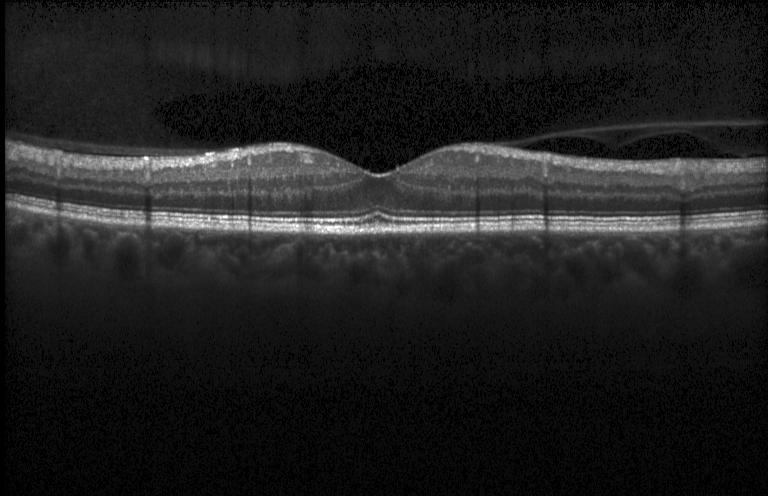

Assessment: no choroidal neovascularization, no diabetic macular edema, and no drusen.